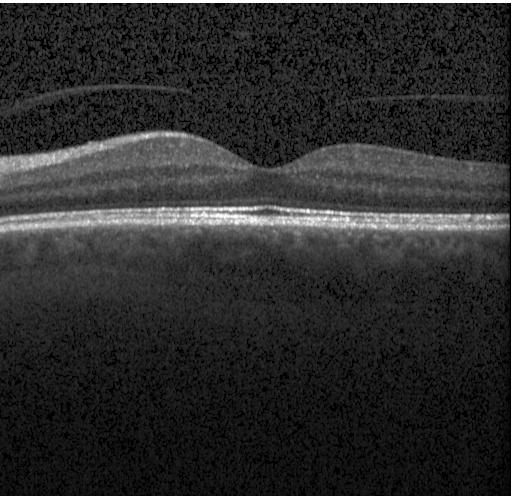 Optical coherence tomography scan
The scan shows no choroidal neovascularization, diabetic macular edema, or drusen.